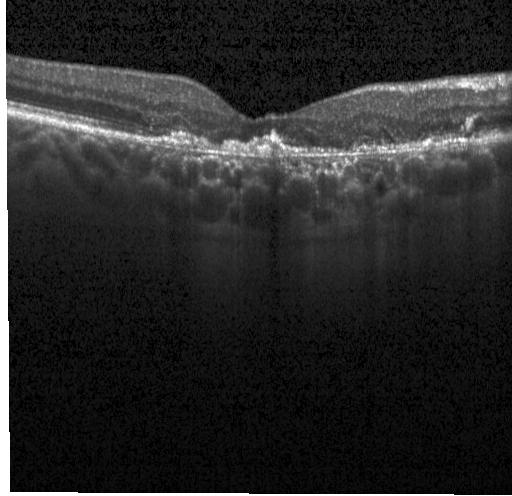

The scan shows a choroidal neovascular membrane.